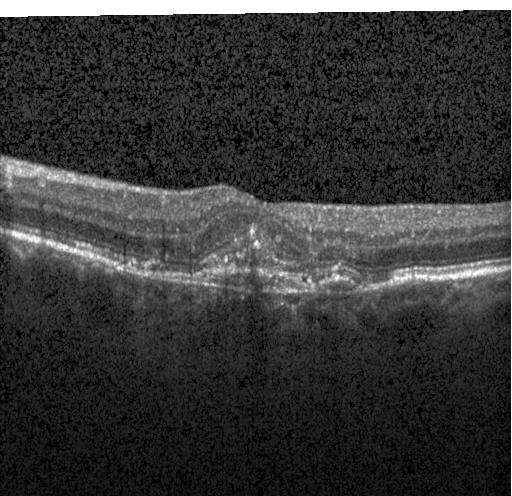
OCT B-scan.
Macular OCT: CNV.